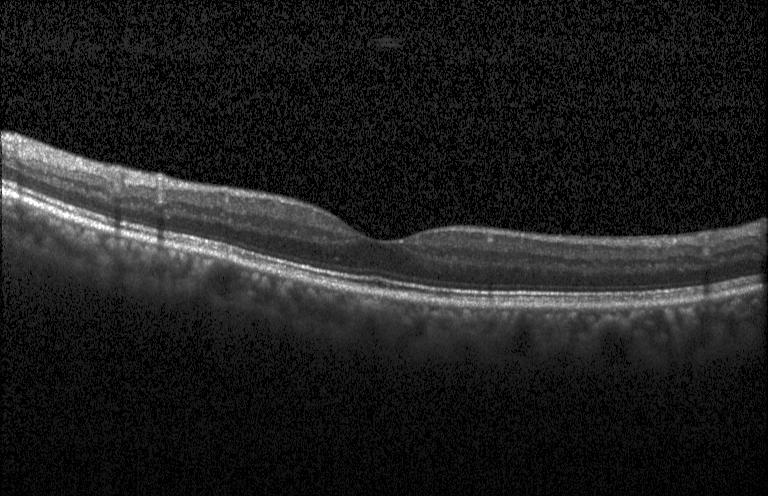 Retinal OCT cross-section. Instrument: Heidelberg Spectralis. Spectral-domain optical coherence tomography. Centered on the fovea. Finding: no choroidal neovascularization, diabetic macular edema, or drusen.